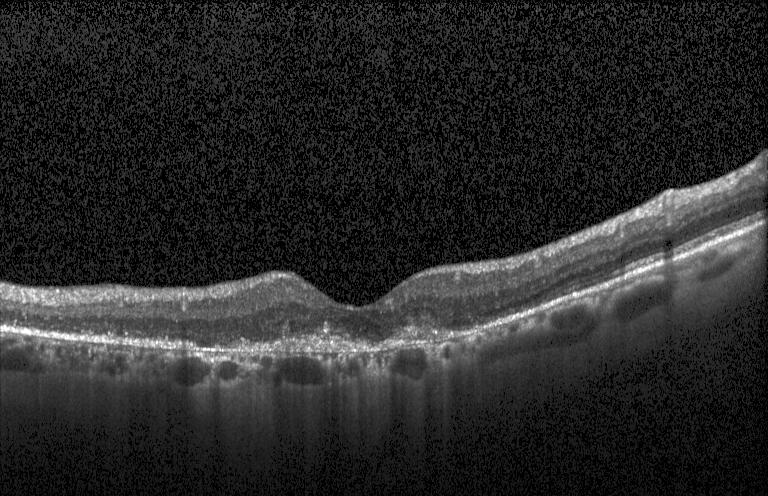 Diagnosis: a choroidal neovascular membrane.